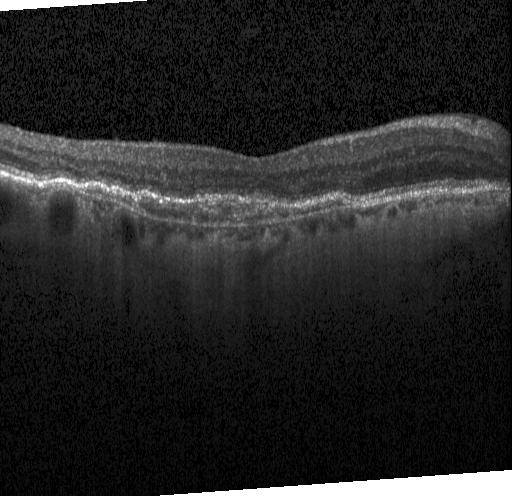 SD-OCT. Horizontal scan through the fovea. Instrument: Heidelberg Spectralis. Optical coherence tomography scan
Impression: choroidal neovascularization.